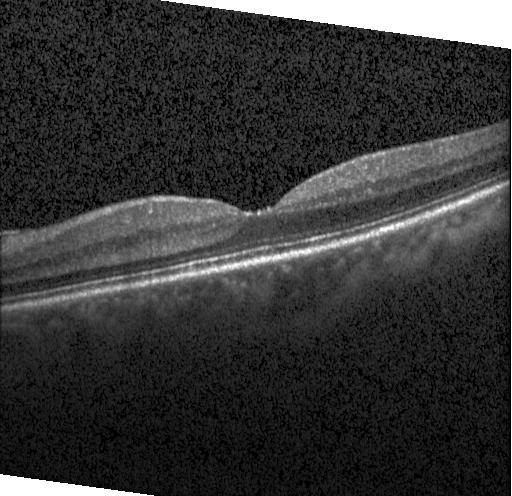 OCT line scan.
OCT finding: no choroidal neovascularization, no diabetic macular edema, and no drusen.